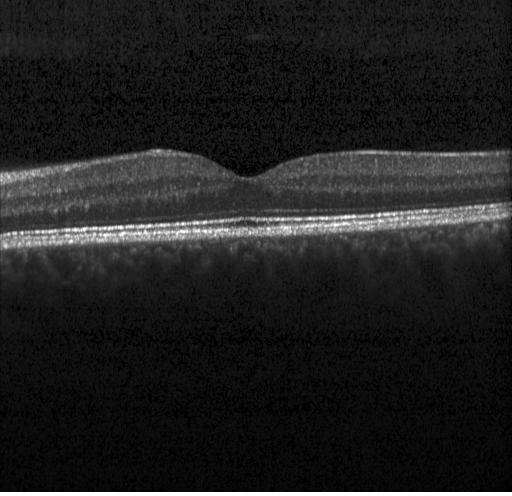

Assessment: no choroidal neovascularization, no diabetic macular edema, and no drusen.